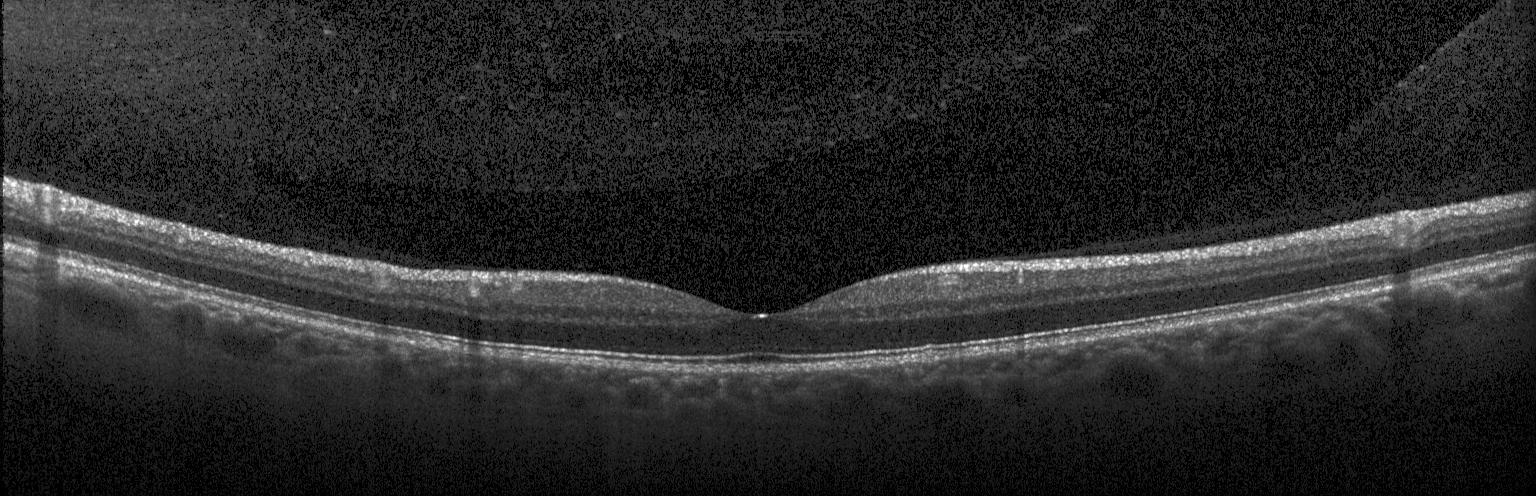

Macular OCT demonstrating no evidence of CNV, DME, or drusen.